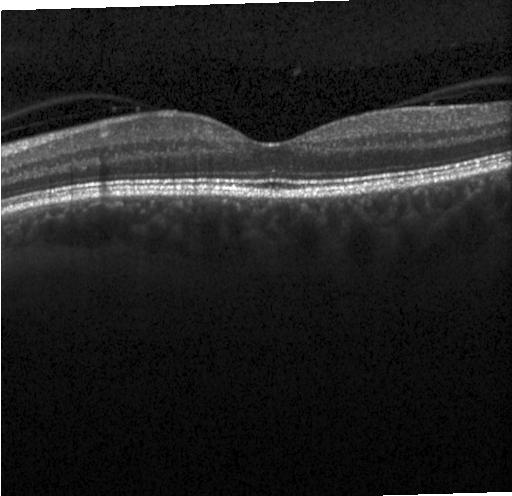
Diagnosis: no evidence of choroidal neovascularization, diabetic macular edema, or drusen.